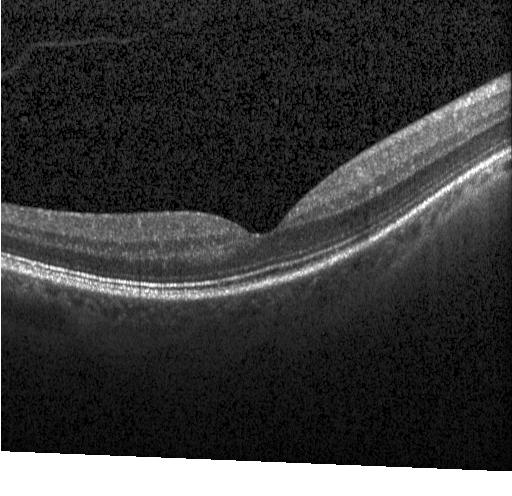
OCT line scan — Finding: neither choroidal neovascularization, diabetic macular edema, nor drusen.